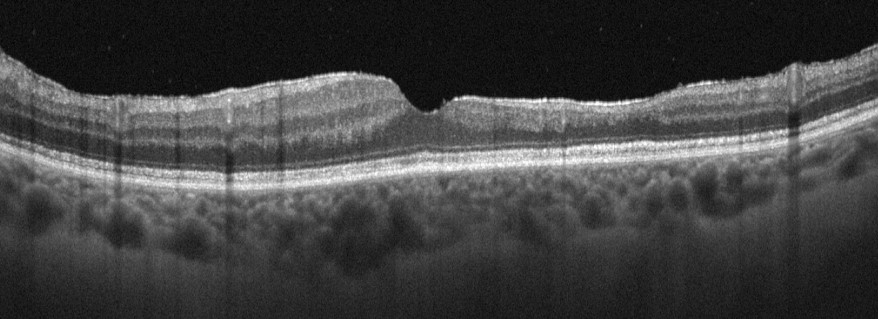

Instrument: Optovue Avanti RTVue XR; retinal OCT cross-section; fovea-centered.
Retinal vein occlusion (RVO).